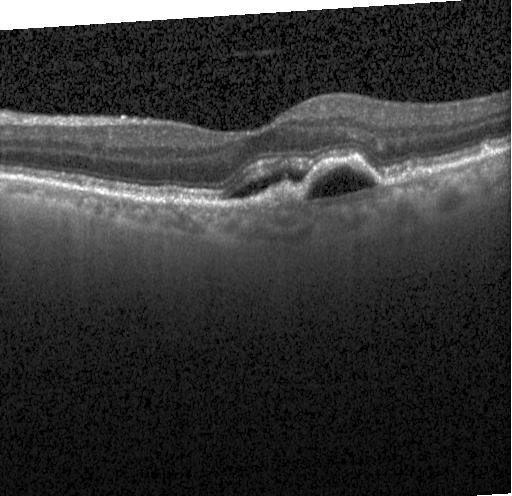

Finding: choroidal neovascularization.